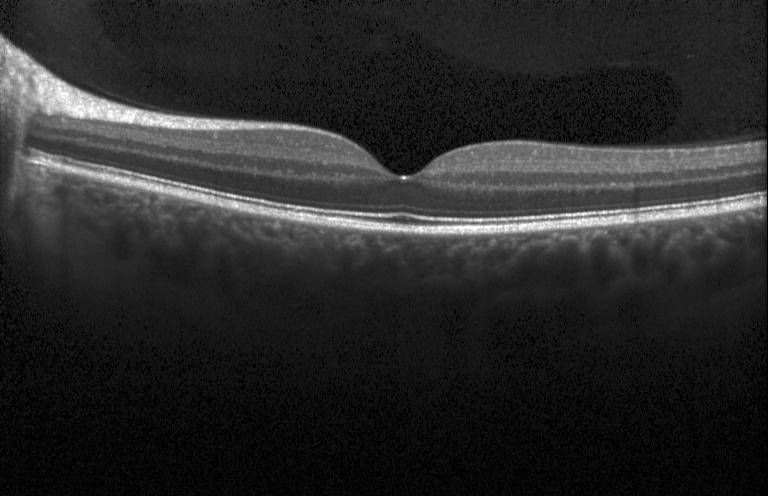 Optical coherence tomography B-scan
Finding: no choroidal neovascularization, diabetic macular edema, or drusen.